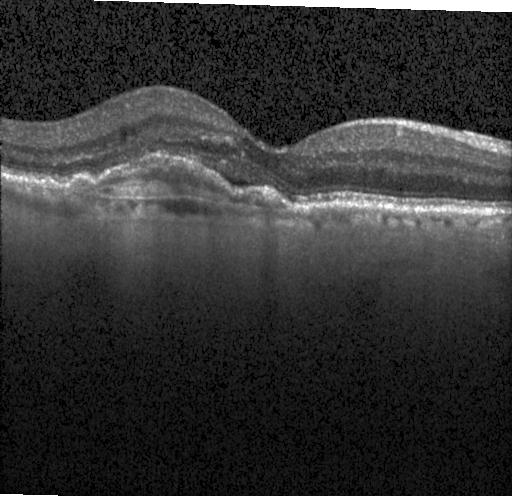 This B-scan demonstrates choroidal neovascularization (CNV).